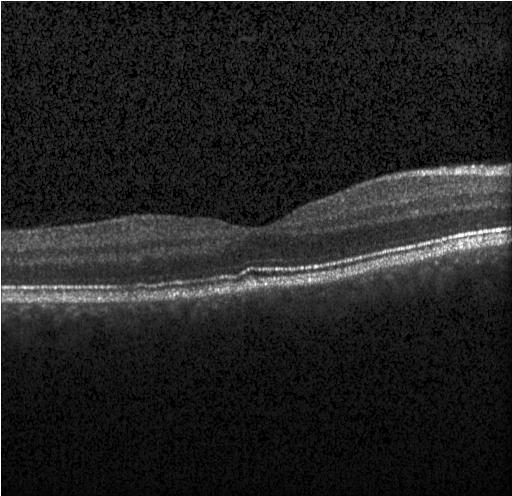

Macular OCT demonstrating no evidence of CNV, DME, or drusen.